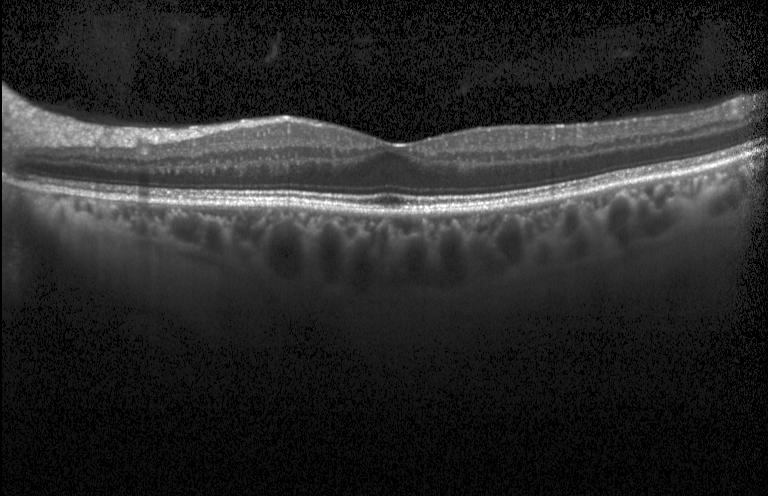
Impression: neither choroidal neovascularization, diabetic macular edema, nor drusen.